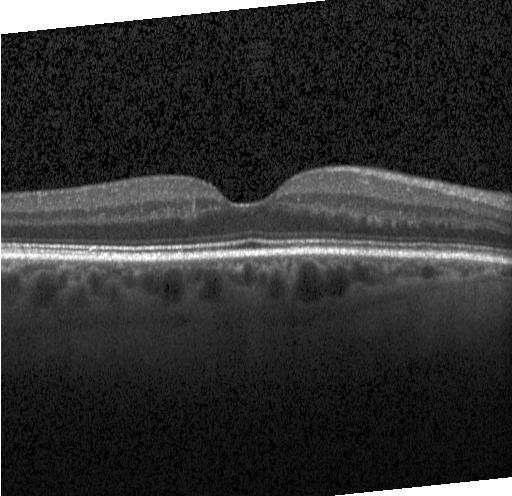
OCT B-scan showing no CNV, DME, or drusen.